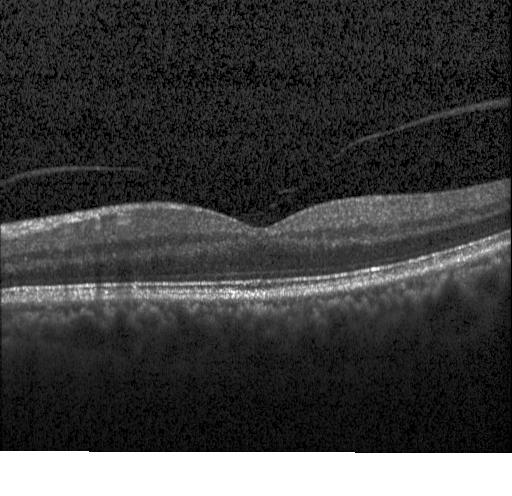

Heidelberg Spectralis; optical coherence tomography scan; SD-OCT; centered on the fovea
Finding: no evidence of choroidal neovascularization, diabetic macular edema, or drusen.